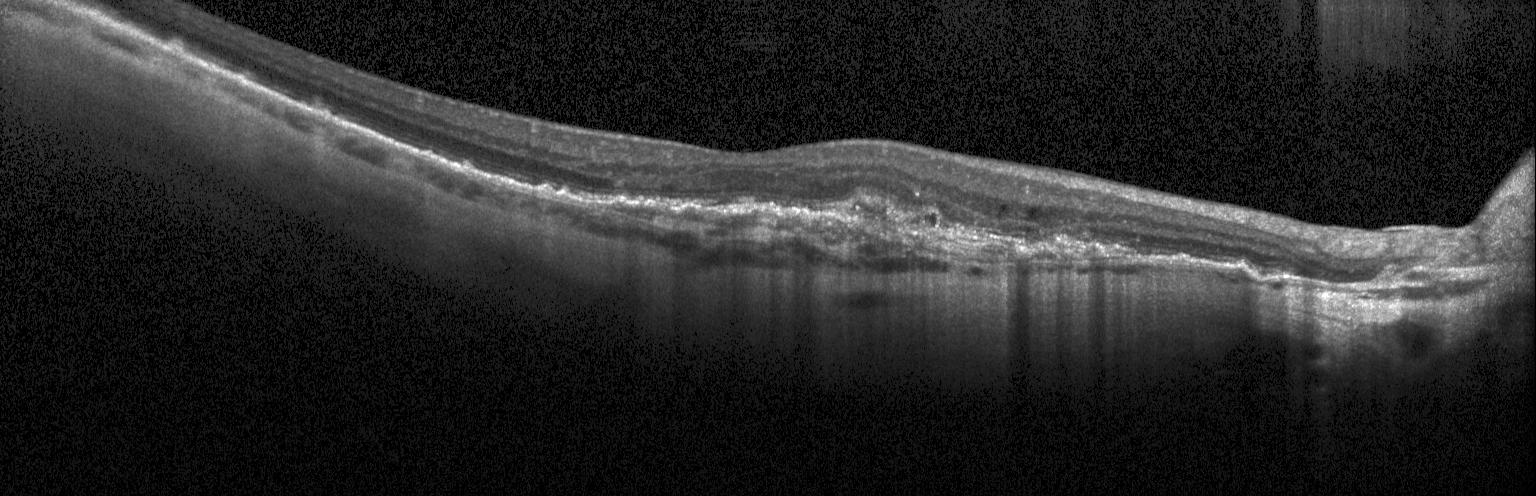 Acquired on a Heidelberg Spectralis; retinal OCT cross-section; spectral-domain optical coherence tomography; macular scan.
Finding: a choroidal neovascular membrane.